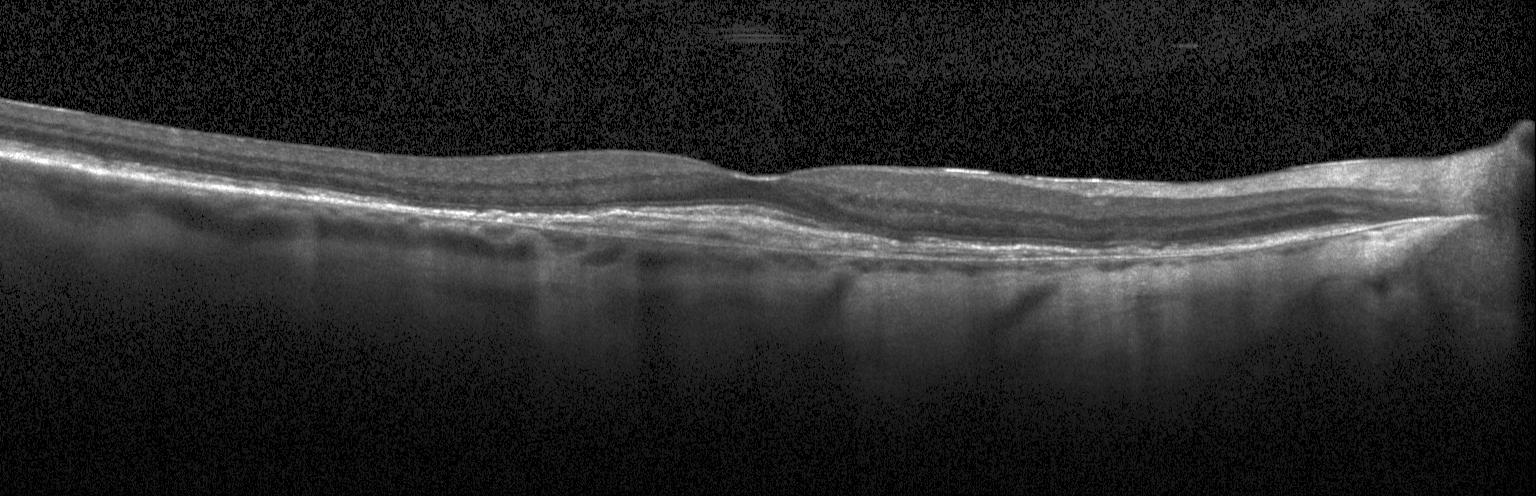

OCT line scan, spectral-domain OCT
Assessment: choroidal neovascularization.